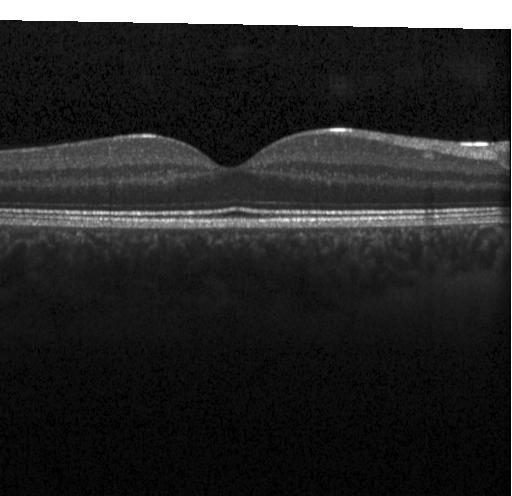 Retinal OCT B-scan.
Dx: no choroidal neovascularization, diabetic macular edema, or drusen.